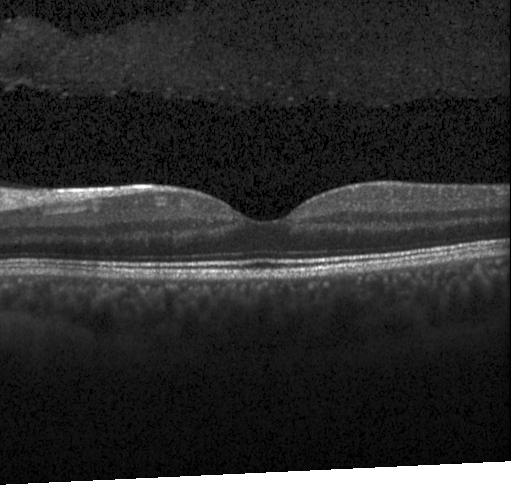

Instrument: Heidelberg Spectralis. Centered on the fovea. Spectral-domain optical coherence tomography. Optical coherence tomography scan — Diagnosis: no CNV, DME, or drusen.